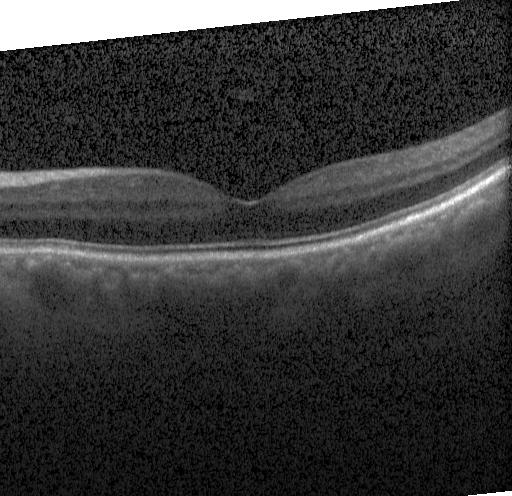 Heidelberg Spectralis. Retinal OCT B-scan. The scan shows no CNV, DME, or drusen.